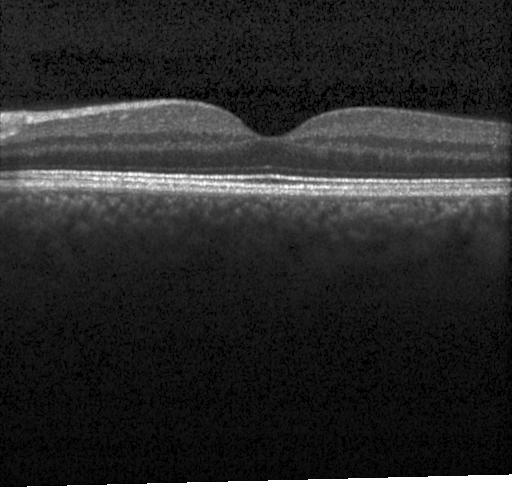
Retinal OCT B-scan; horizontal scan through the fovea; Heidelberg Spectralis; spectral-domain OCT
OCT finding: no evidence of choroidal neovascularization, diabetic macular edema, or drusen.